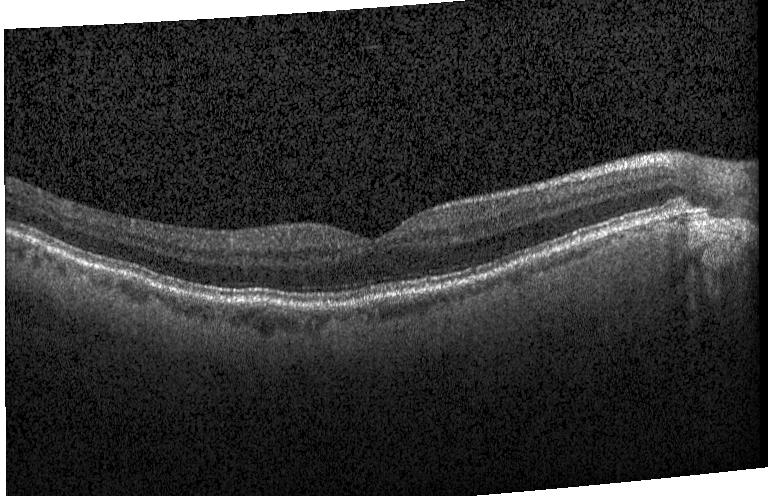 Macular OCT demonstrating no choroidal neovascularization, no diabetic macular edema, and no drusen.